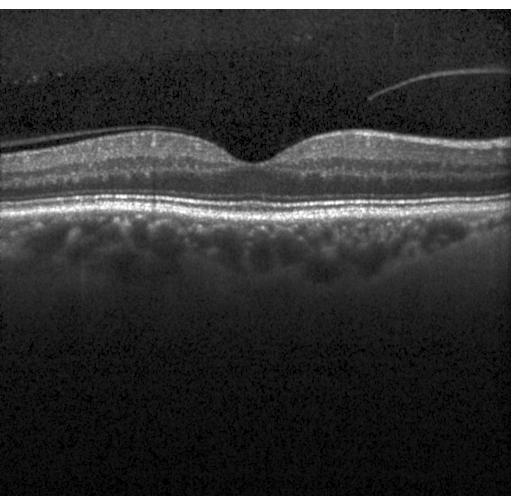

Dx: no CNV, no DME, and no drusen.